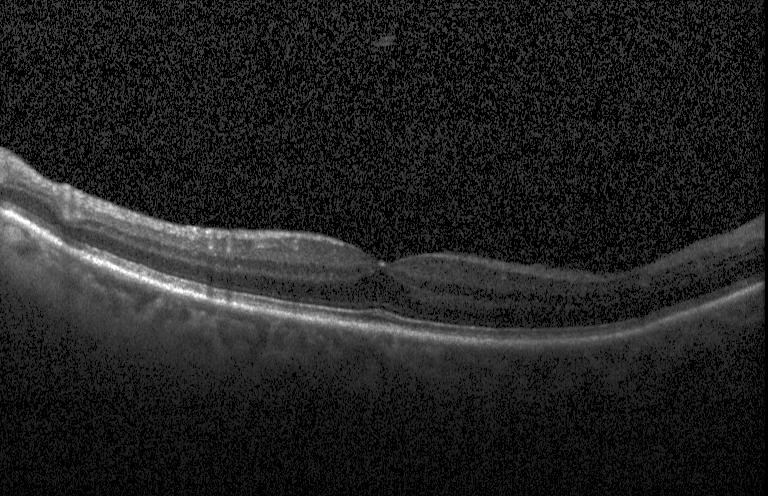

The scan shows neither choroidal neovascularization, diabetic macular edema, nor drusen.